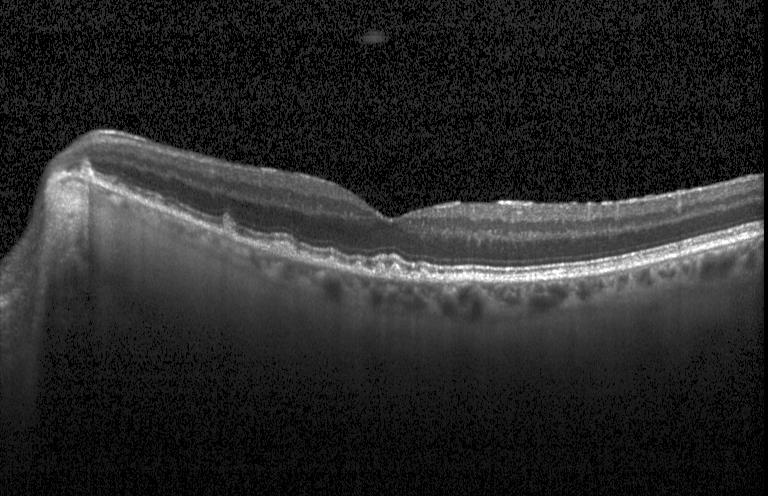
Macular OCT: drusen.